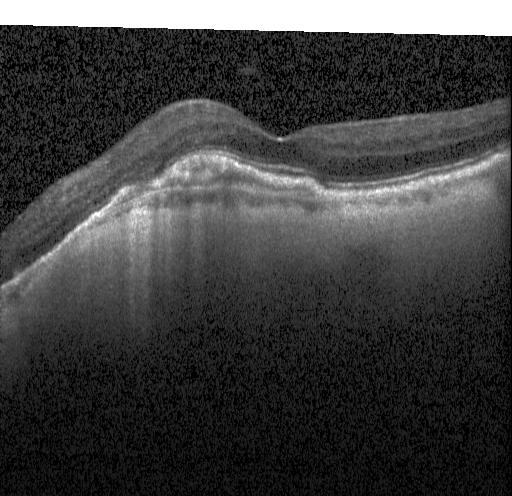
Acquired on a Heidelberg Spectralis. Centered on the fovea. Optical coherence tomography scan — Impression: a choroidal neovascular membrane.